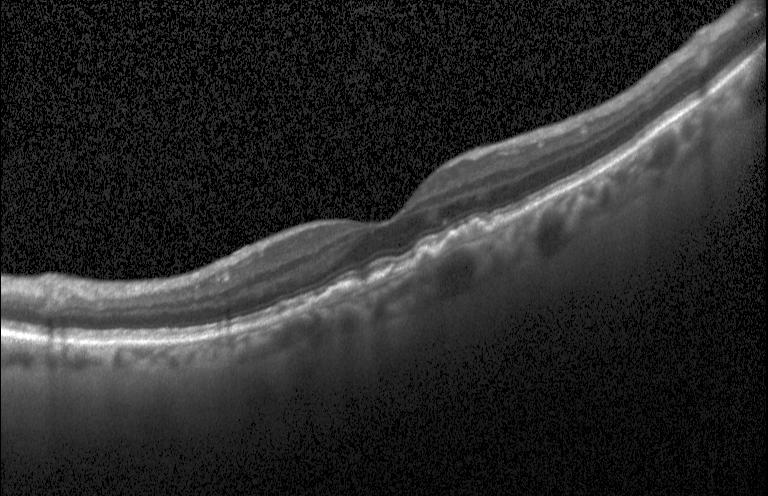

Optical coherence tomography B-scan — Finding: a choroidal neovascular membrane.